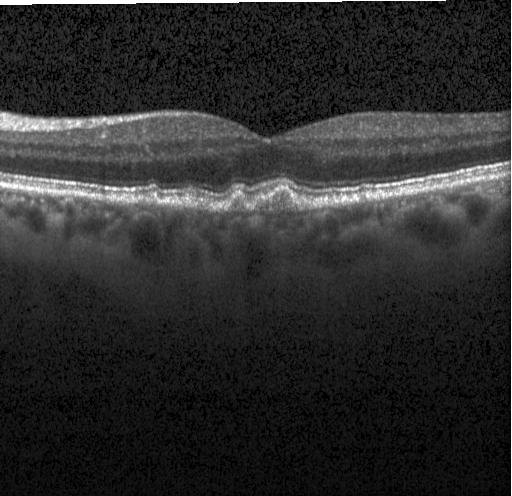
Optical coherence tomography B-scan — Finding: multiple drusen.